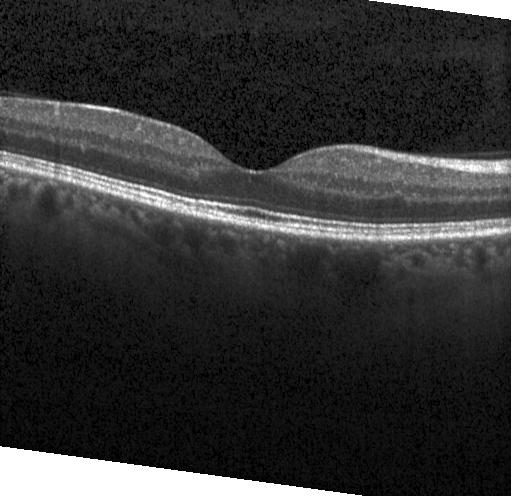

Spectral-domain optical coherence tomography. Macular scan. OCT line scan. Heidelberg Spectralis OCT system. Dx: no evidence of choroidal neovascularization, diabetic macular edema, or drusen.